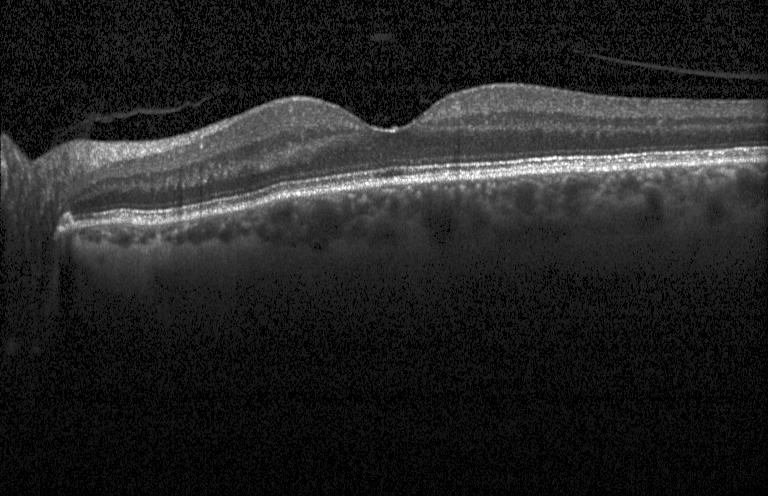
The scan shows neither choroidal neovascularization, diabetic macular edema, nor drusen.